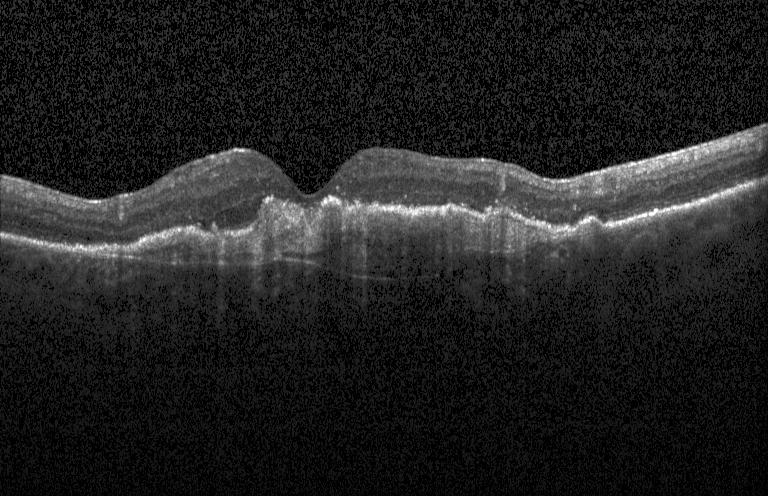

Through the macula · retinal OCT cross-section. Macular OCT: a choroidal neovascular membrane.